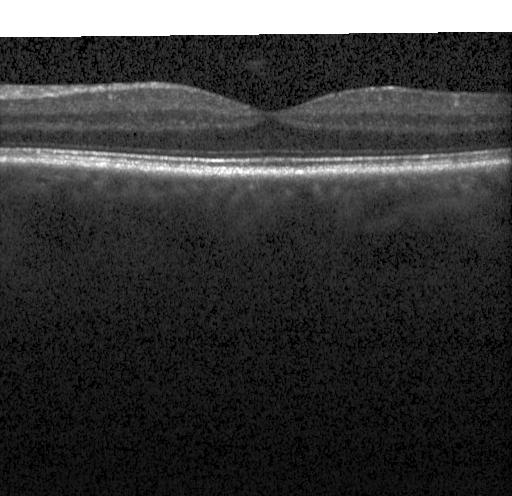 Retinal OCT cross-section
Finding: no evidence of choroidal neovascularization, diabetic macular edema, or drusen.